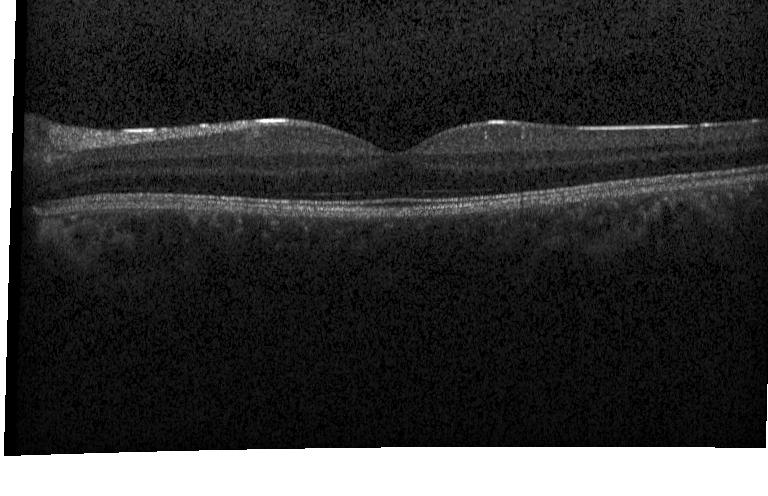
OCT B-scan — Assessment: neither choroidal neovascularization, diabetic macular edema, nor drusen.